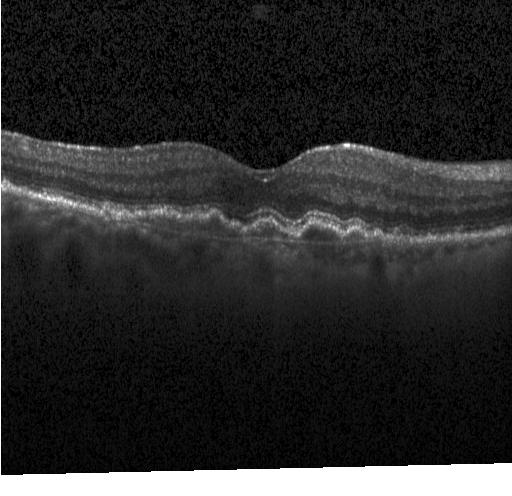
Horizontal scan through the fovea, spectral-domain optical coherence tomography, instrument: Heidelberg Spectralis, retinal OCT cross-section — This B-scan demonstrates CNV.